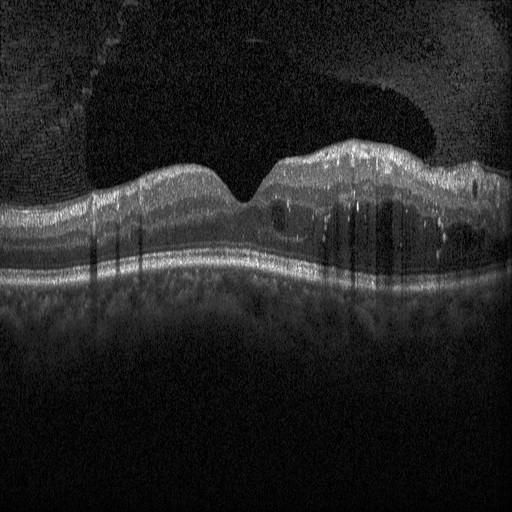

OCT B-scan · macular scan · acquired on a Heidelberg Spectralis — Diagnosis: DME.